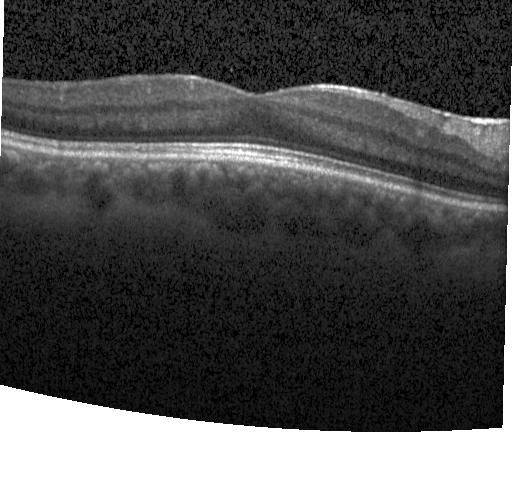 OCT scan showing no evidence of choroidal neovascularization, diabetic macular edema, or drusen.